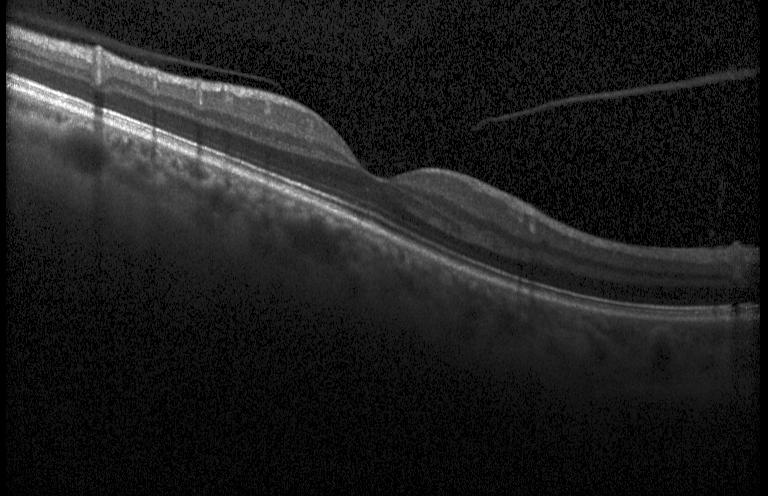
OCT line scan; Heidelberg Spectralis OCT system. This B-scan demonstrates no evidence of choroidal neovascularization, diabetic macular edema, or drusen.